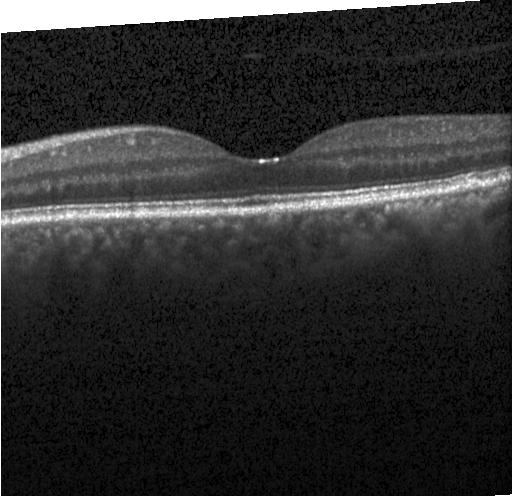

Spectral-domain OCT · OCT line scan — Impression: no evidence of choroidal neovascularization, diabetic macular edema, or drusen.